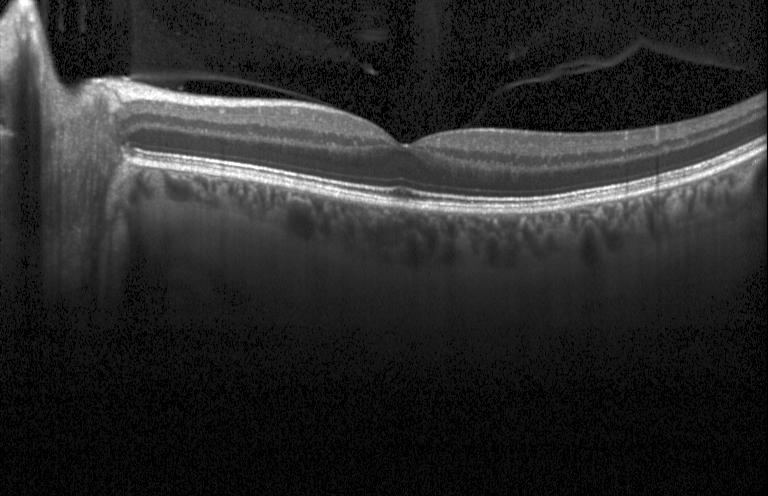

Optical coherence tomography B-scan; fovea-centered; SD-OCT; acquired on a Heidelberg Spectralis
The scan shows no evidence of CNV, DME, or drusen.